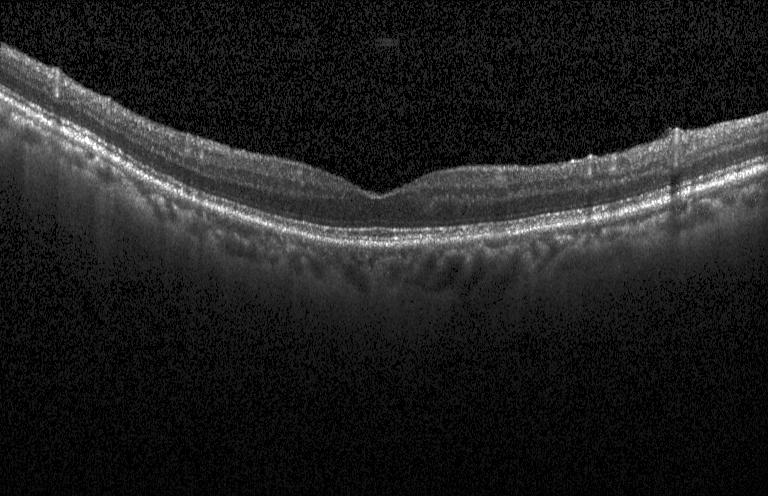
Optical coherence tomography scan.
Impression: no CNV, no DME, and no drusen.